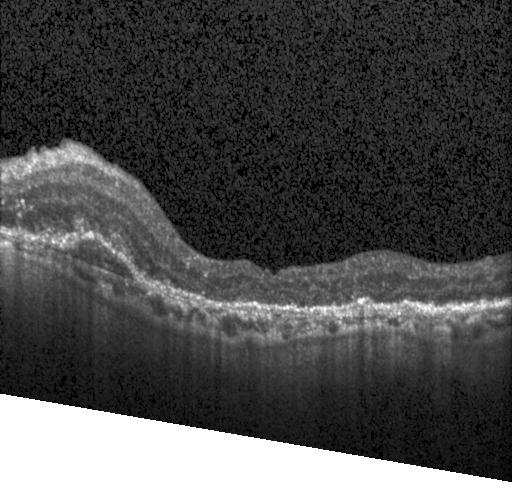

Retinal OCT cross-section.
Impression: choroidal neovascularization (CNV).